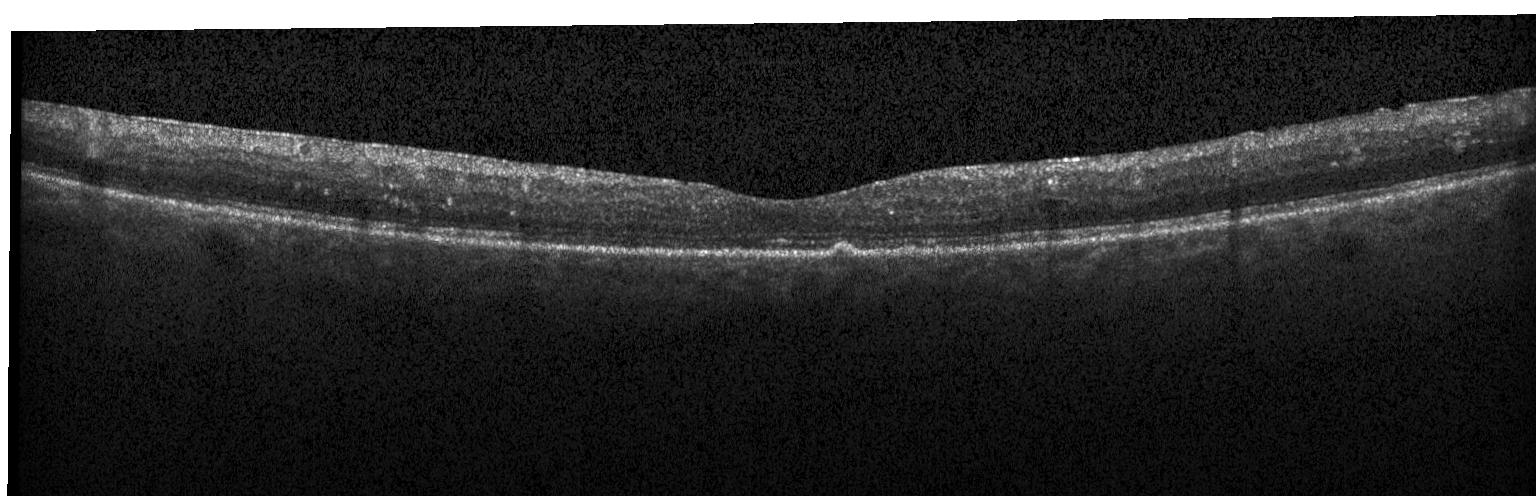

Instrument: Heidelberg Spectralis; spectral-domain OCT; optical coherence tomography B-scan
Finding: multiple drusen.